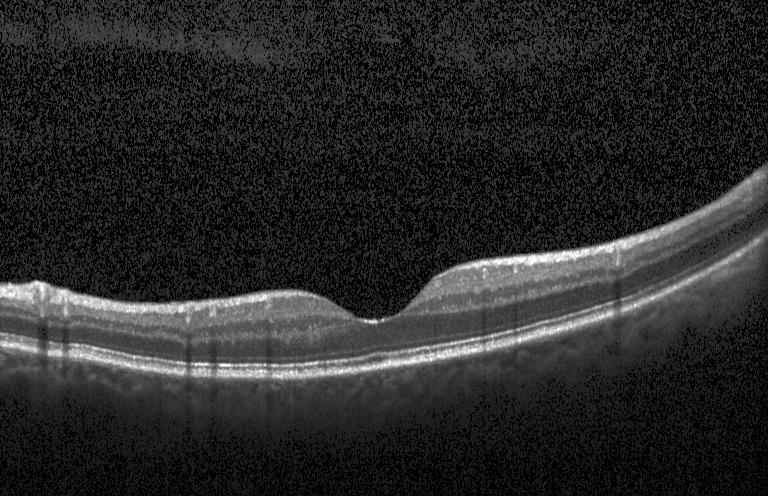 OCT scan showing no evidence of CNV, DME, or drusen.